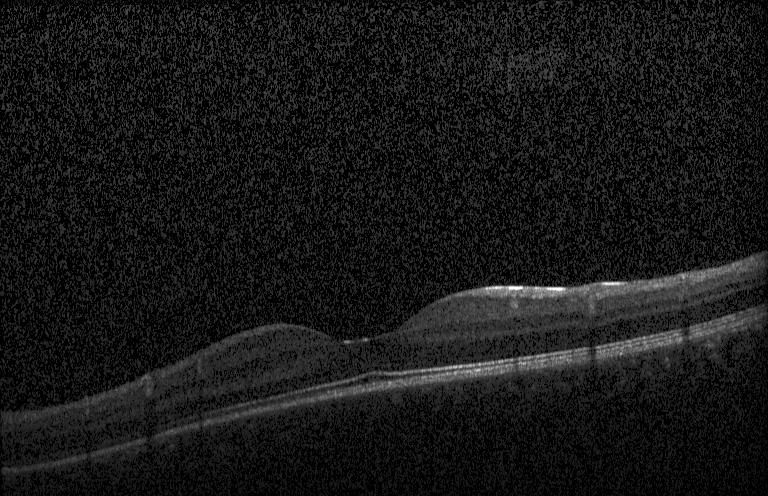 Horizontal scan through the fovea. Optical coherence tomography B-scan. Heidelberg Spectralis OCT system.
Macular OCT: no evidence of choroidal neovascularization, diabetic macular edema, or drusen.